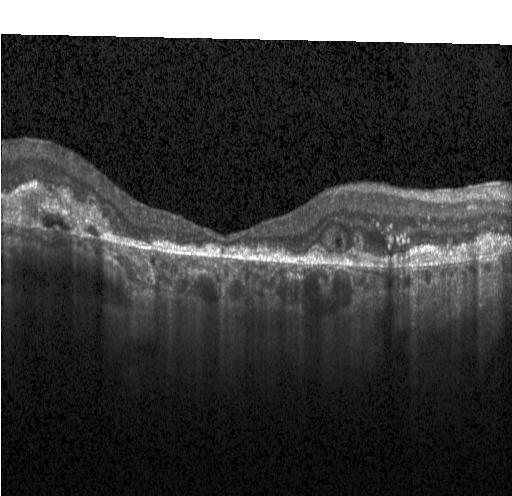

Diagnosis: CNV.